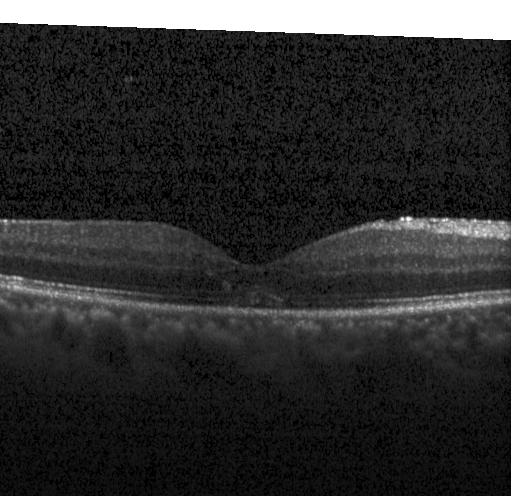 Dx: no evidence of choroidal neovascularization, diabetic macular edema, or drusen.